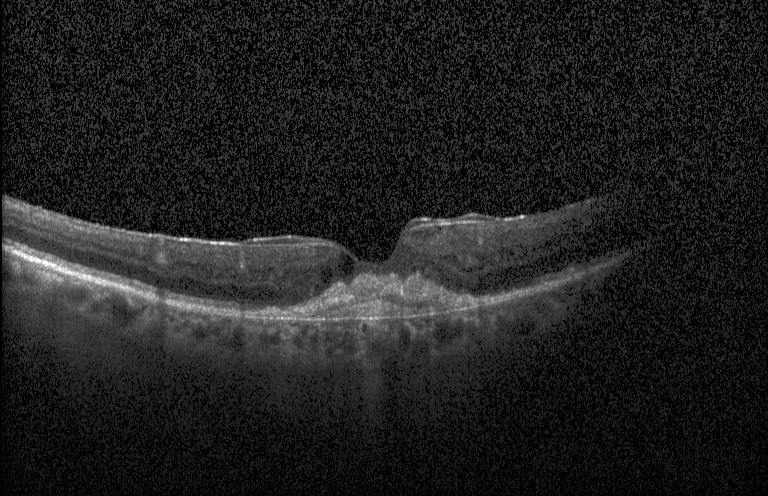

Retinal OCT cross-section showing CNV.